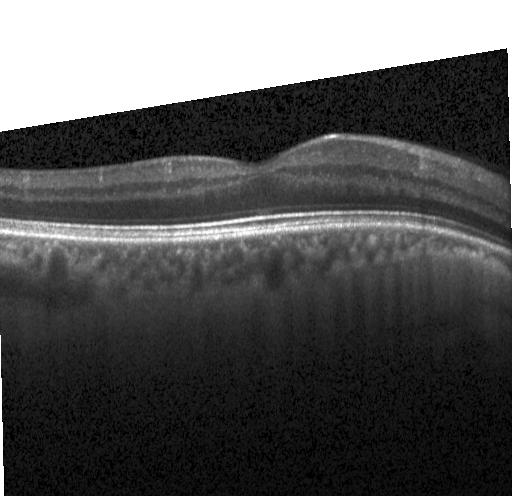 This B-scan demonstrates no evidence of CNV, DME, or drusen.